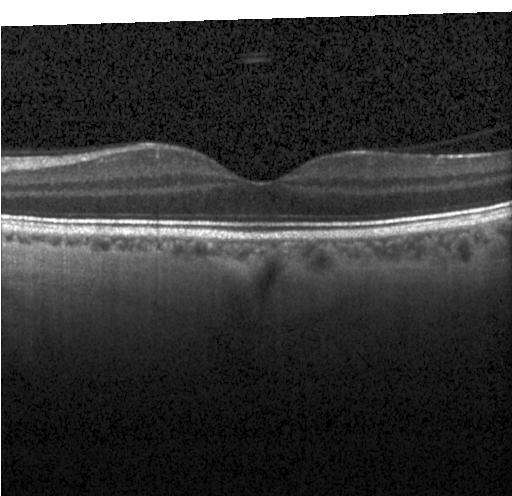 Spectral-domain OCT B-scan: no choroidal neovascularization, no diabetic macular edema, and no drusen.